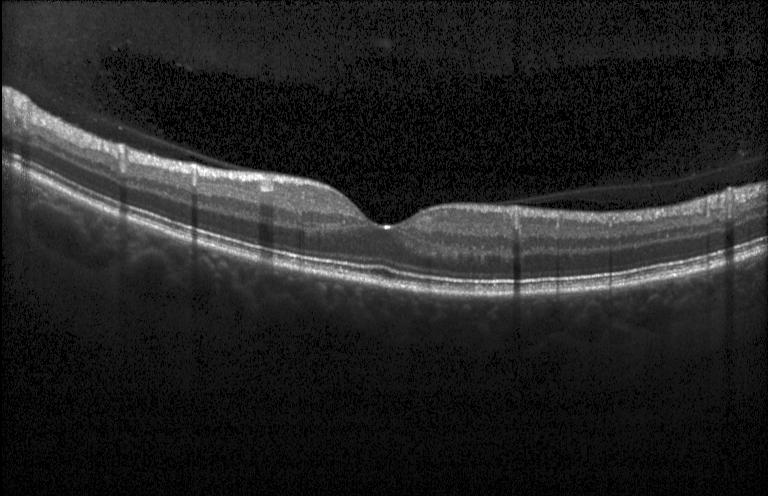
Retinal OCT cross-section showing no choroidal neovascularization, diabetic macular edema, or drusen.